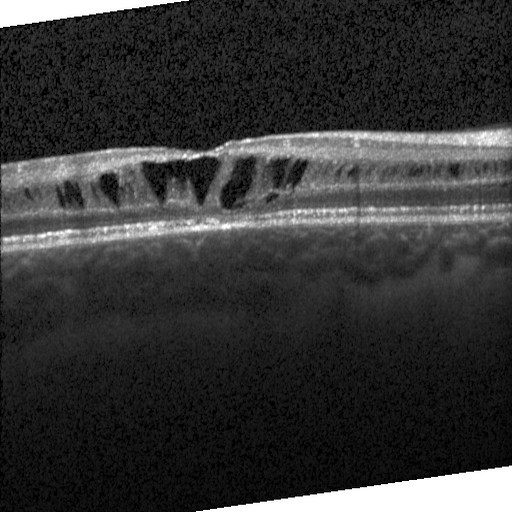 OCT scan showing diabetic macular edema (DME).